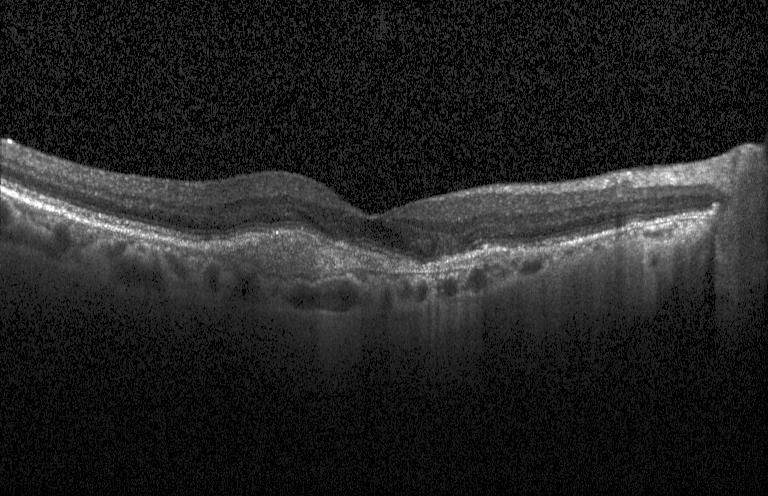 Impression: a choroidal neovascular membrane.